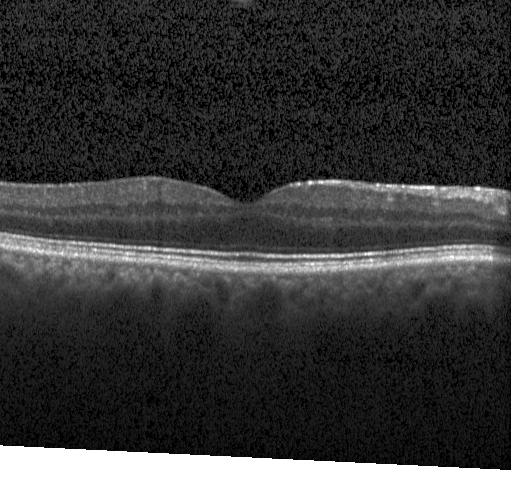
Macular OCT: neither choroidal neovascularization, diabetic macular edema, nor drusen.